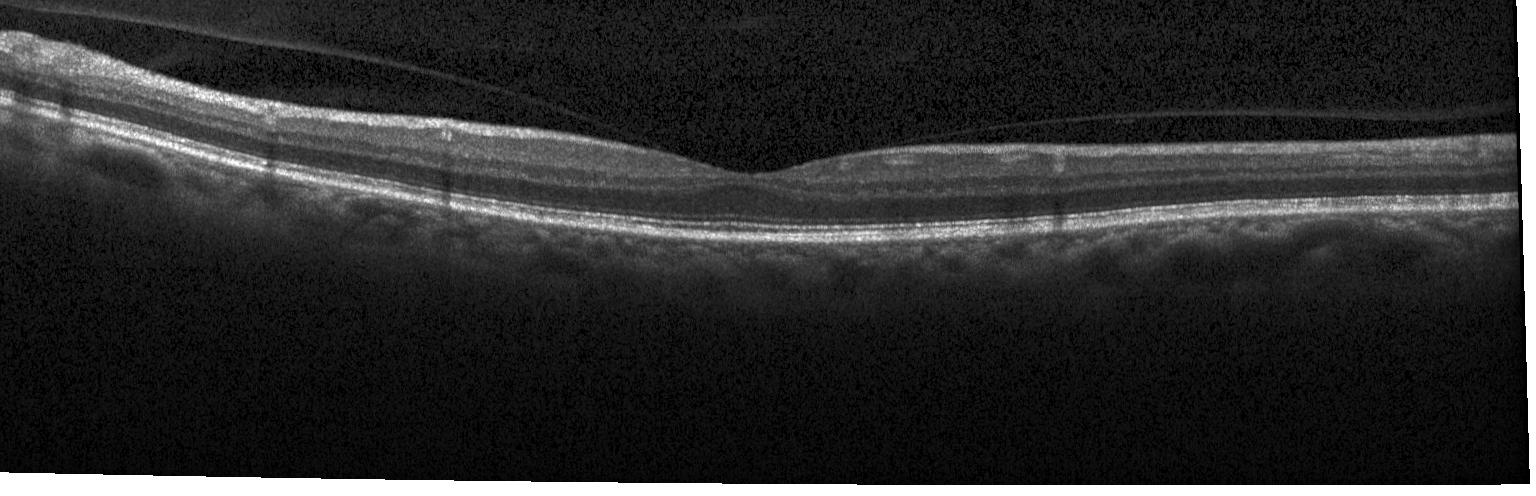

OCT line scan — Impression: no choroidal neovascularization, no diabetic macular edema, and no drusen.